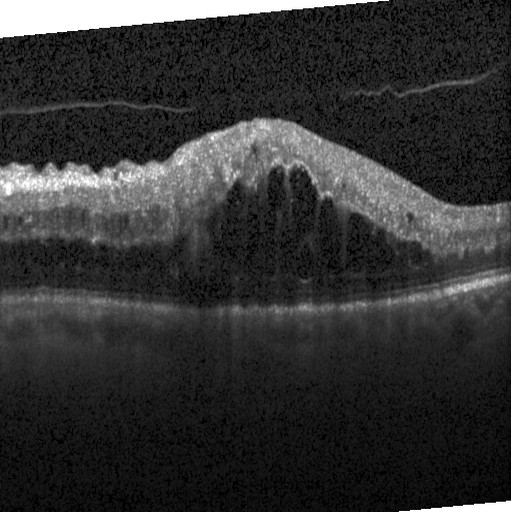
OCT finding: diabetic macular edema (DME).